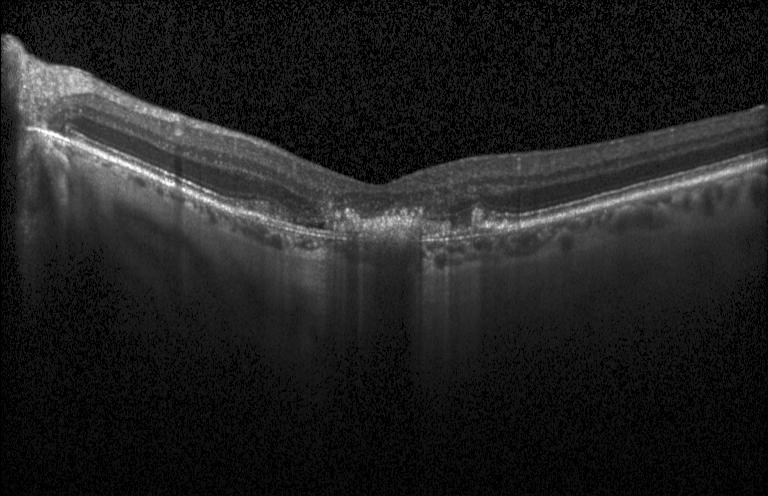
Optical coherence tomography scan; Heidelberg Spectralis; centered on the fovea; spectral-domain optical coherence tomography
Impression: a choroidal neovascular membrane.